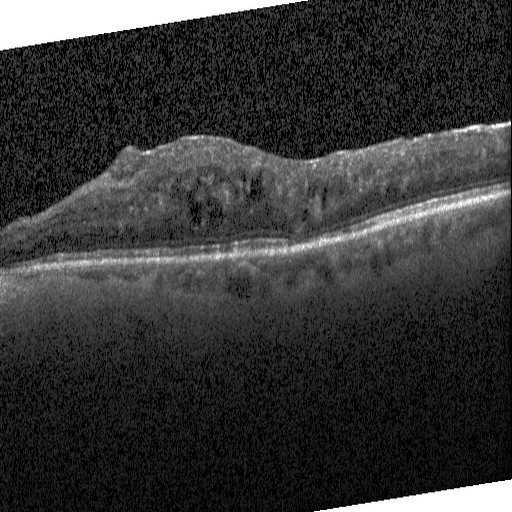 Assessment: diabetic macular edema (DME).